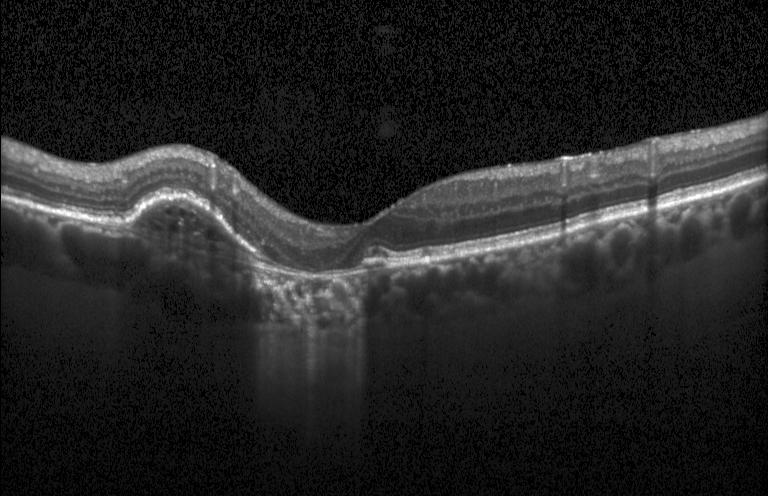
Finding: a choroidal neovascular membrane.